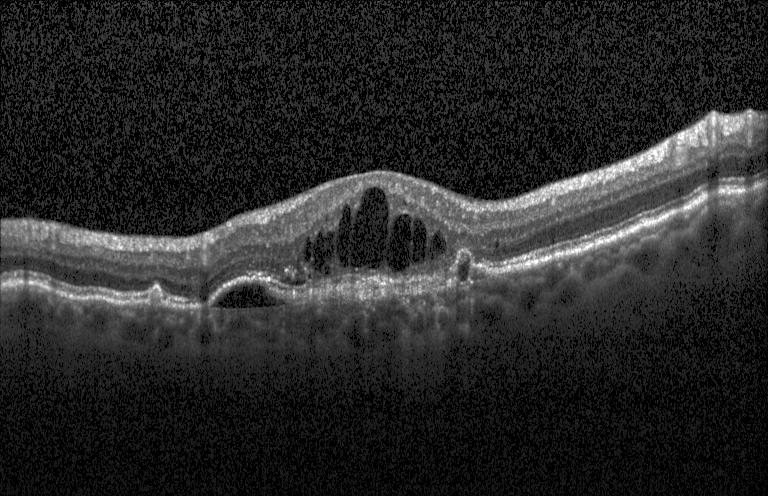

Assessment: choroidal neovascularization (CNV).